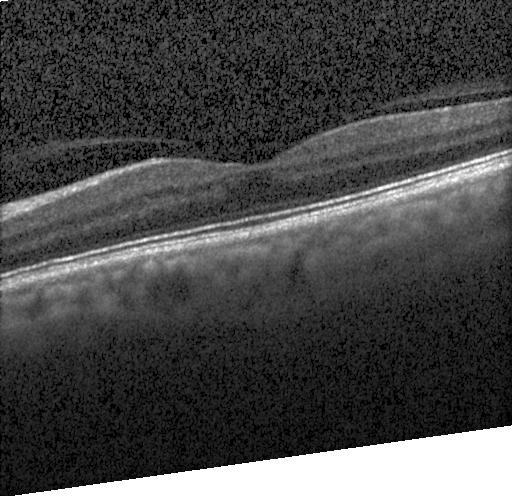
Dx: no CNV, no DME, and no drusen.